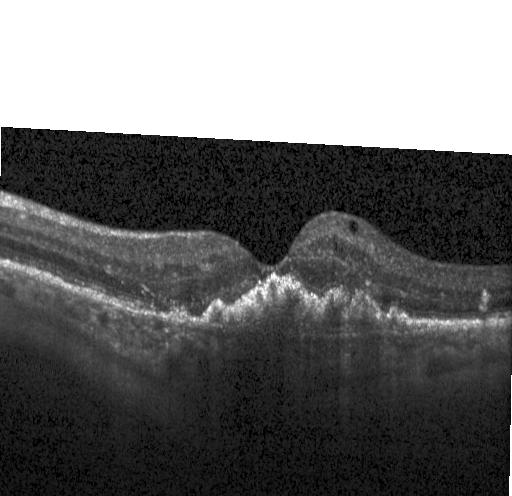 Retinal OCT cross-section — CNV.